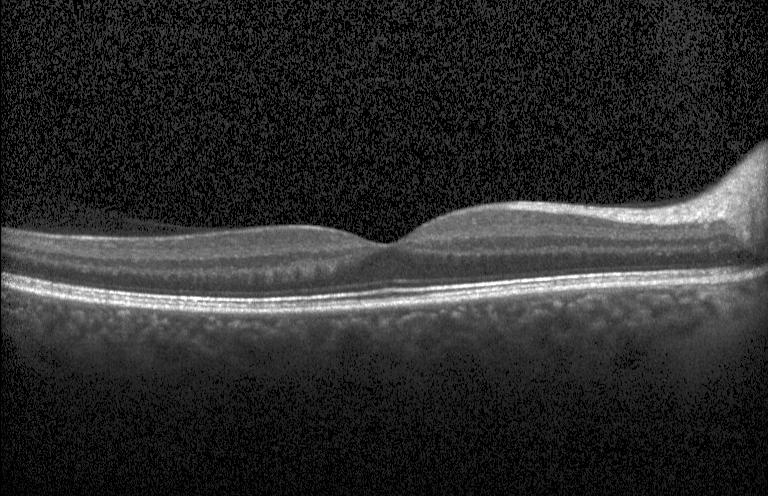
Horizontal scan through the fovea, acquired on a Heidelberg Spectralis, optical coherence tomography B-scan. Macular OCT: no CNV, DME, or drusen.